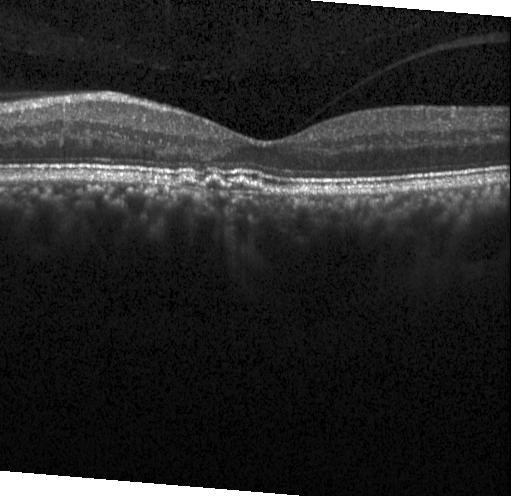
Optical coherence tomography B-scan — Assessment: multiple drusen.